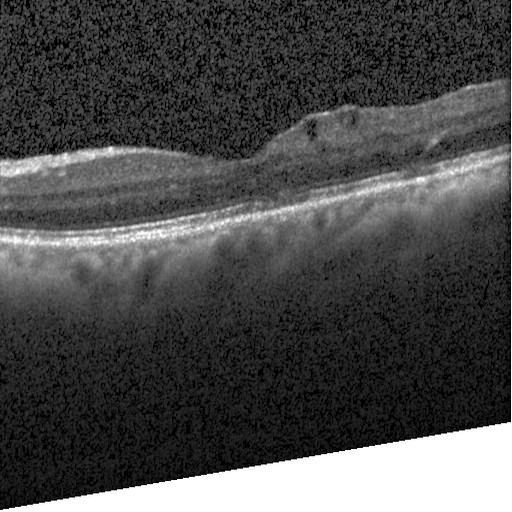 Instrument: Heidelberg Spectralis. Horizontal scan through the fovea. SD-OCT. Retinal OCT cross-section
Diagnosis: diabetic macular edema (DME).